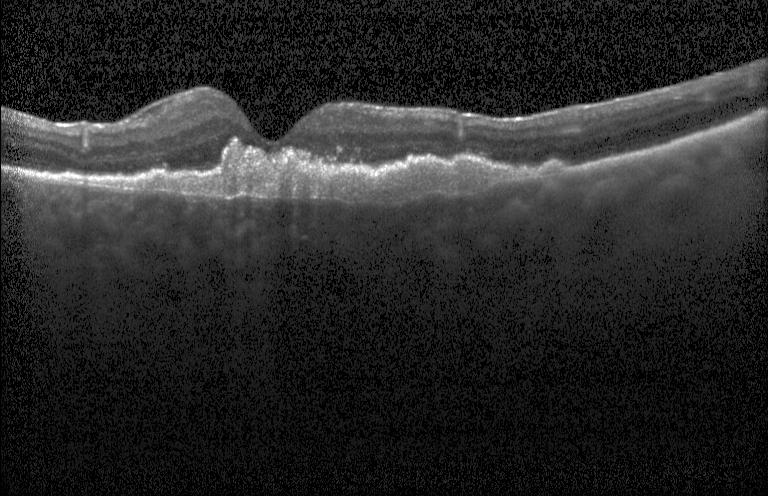 Optical coherence tomography scan · macular scan · SD-OCT. OCT finding: CNV.